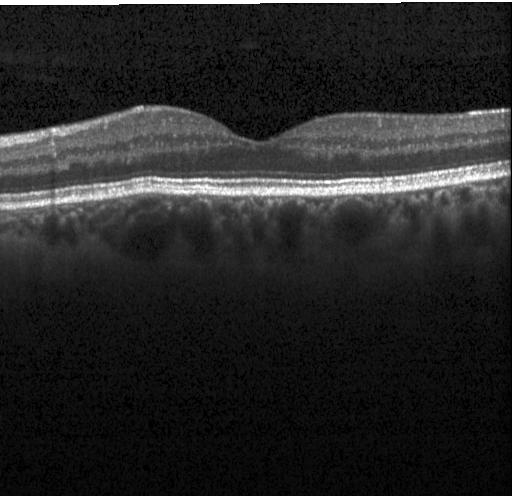
Diagnosis: no choroidal neovascularization, diabetic macular edema, or drusen.